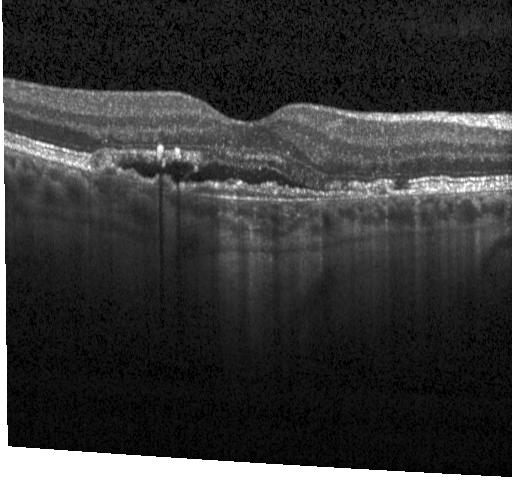

Retinal OCT cross-section showing choroidal neovascularization.